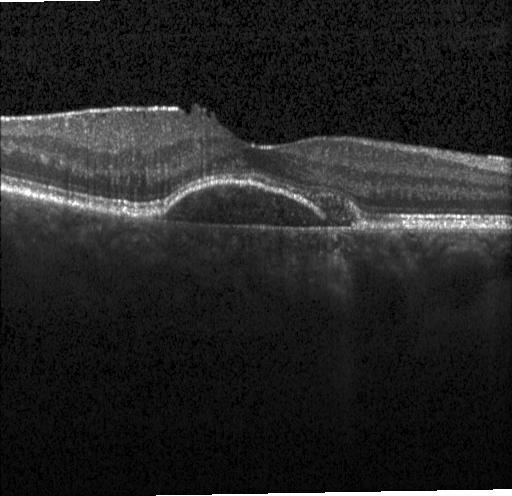

Impression: a choroidal neovascular membrane.